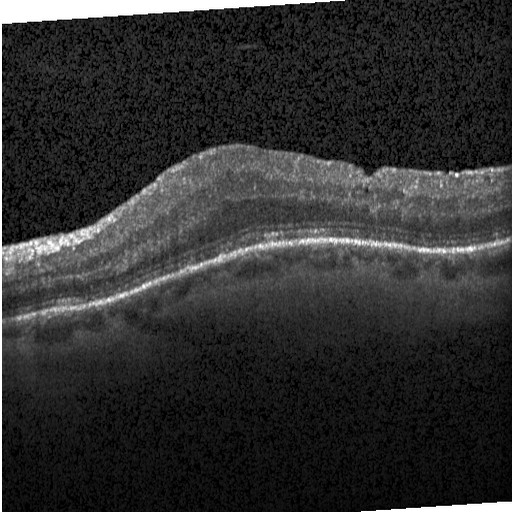 Impression: DME.